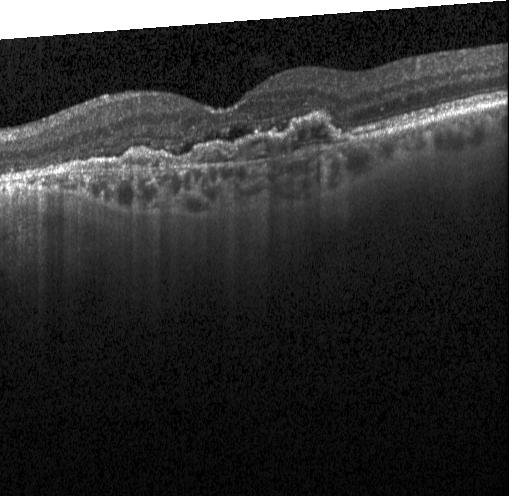
Retinal OCT cross-section.
This B-scan demonstrates a choroidal neovascular membrane.